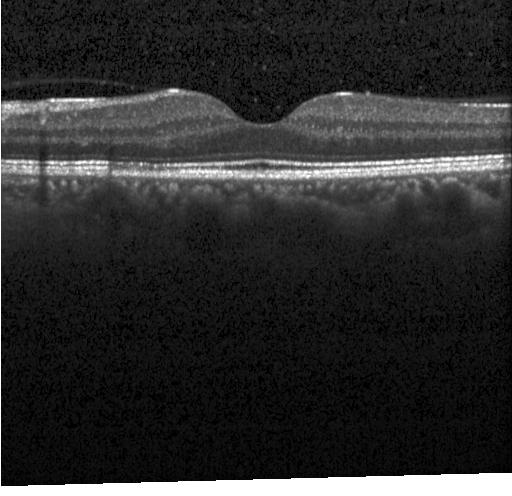

Heidelberg Spectralis. OCT line scan. Spectral-domain optical coherence tomography. Fovea-centered. This B-scan demonstrates no CNV, DME, or drusen.